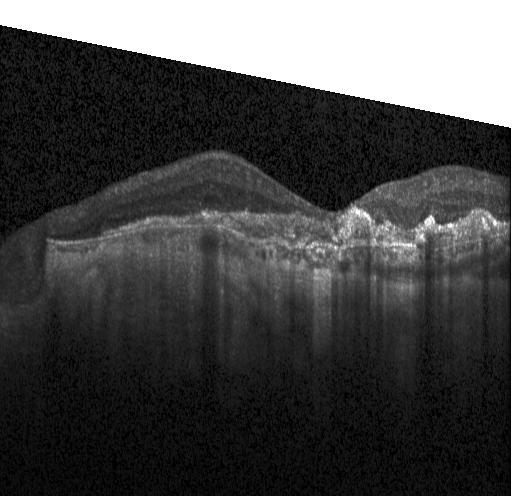 Optical coherence tomography B-scan
Impression: a choroidal neovascular membrane.